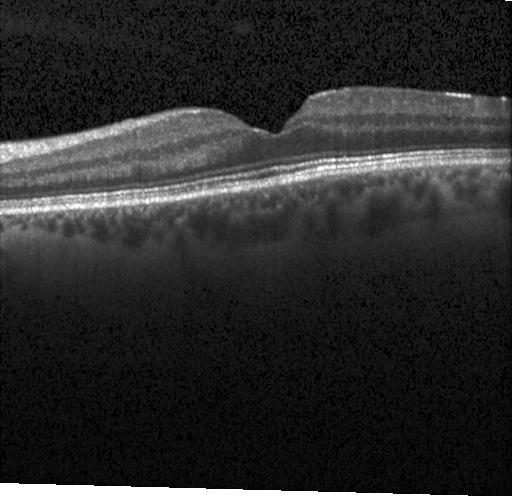 OCT line scan
Diagnosis: no evidence of choroidal neovascularization, diabetic macular edema, or drusen.